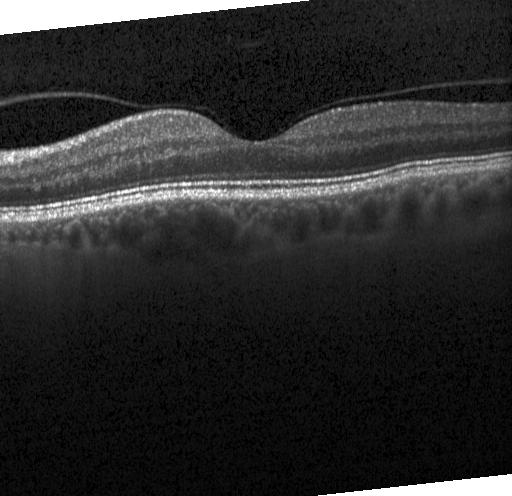 Retinal OCT B-scan. Diagnosis: no choroidal neovascularization, no diabetic macular edema, and no drusen.